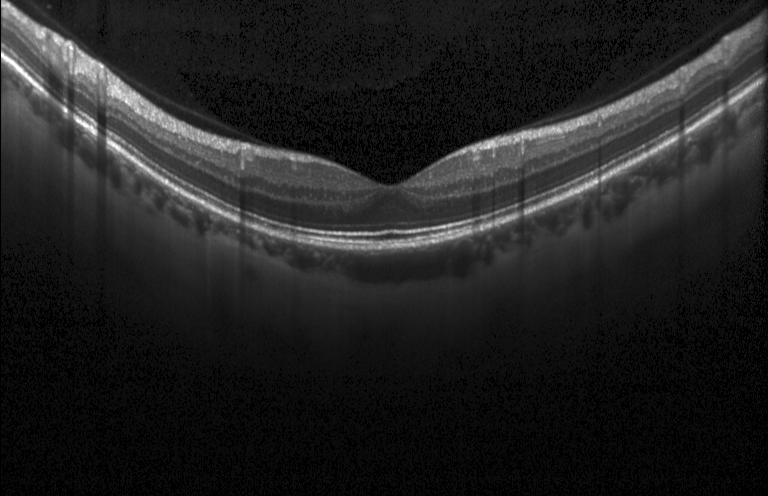 Spectral-domain OCT B-scan: no choroidal neovascularization, no diabetic macular edema, and no drusen.